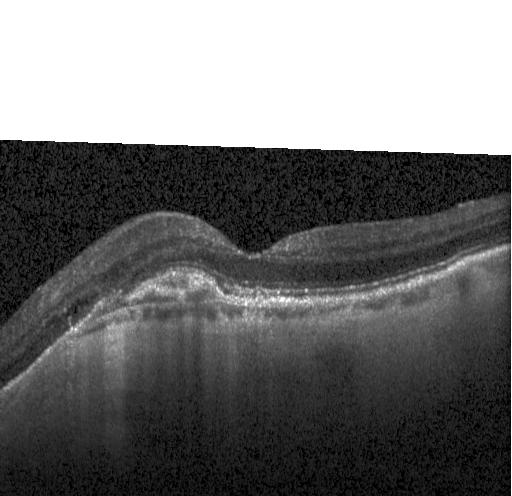

OCT B-scan showing a choroidal neovascular membrane.